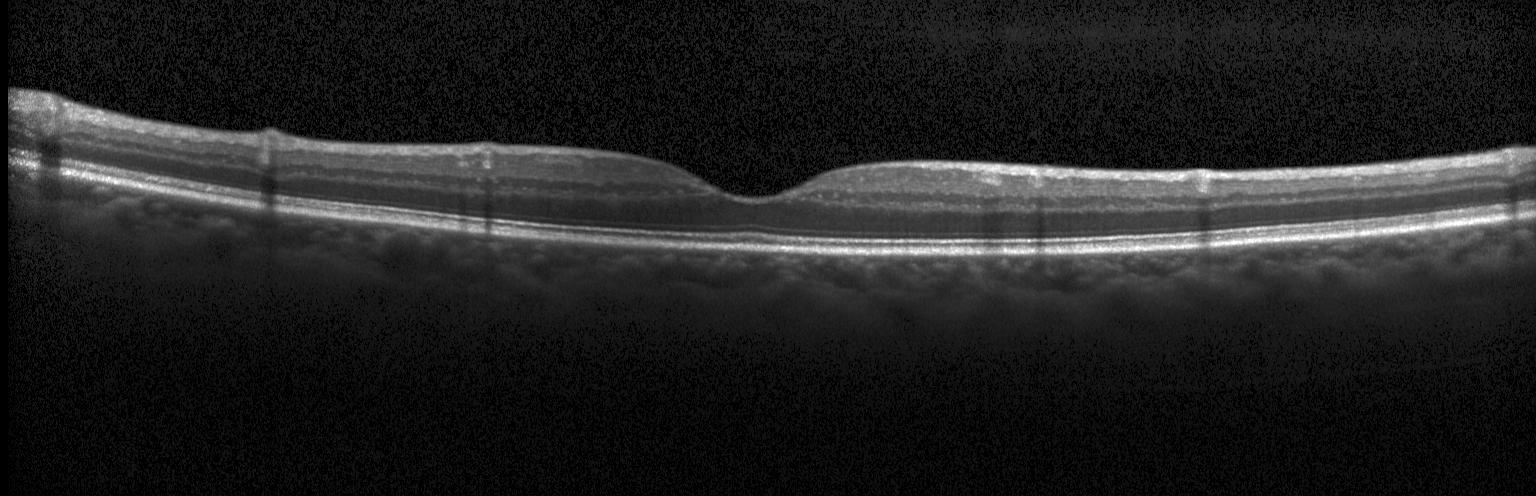

Retinal OCT cross-section; SD-OCT; through the macula. Macular OCT: neither choroidal neovascularization, diabetic macular edema, nor drusen.